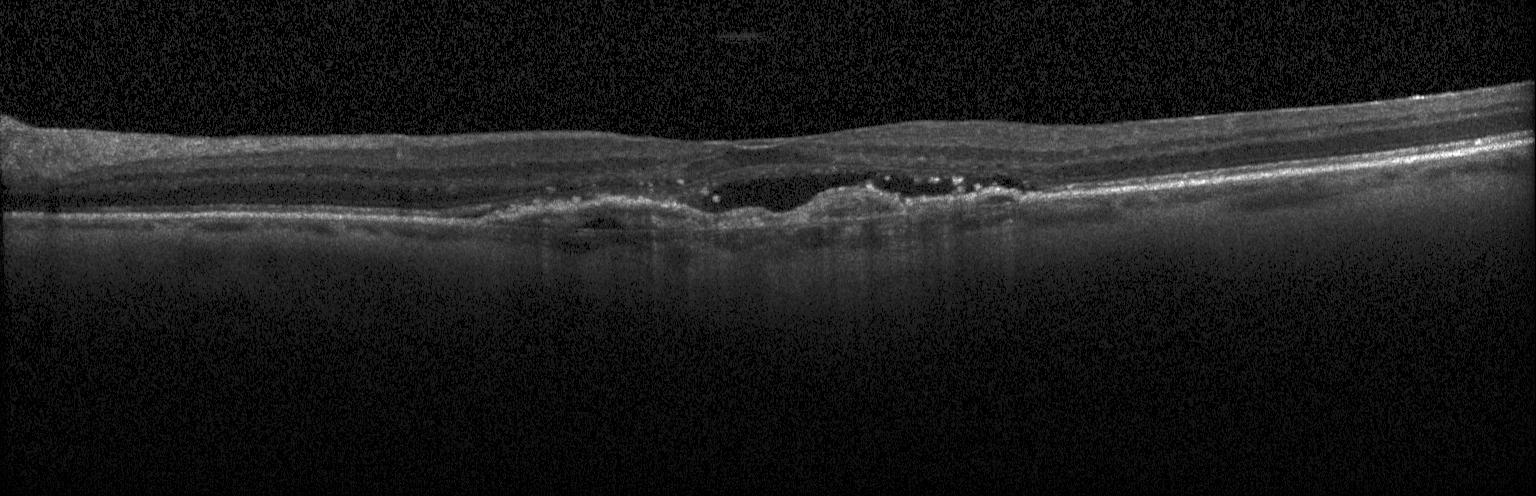 Optical coherence tomography B-scan.
A choroidal neovascular membrane.